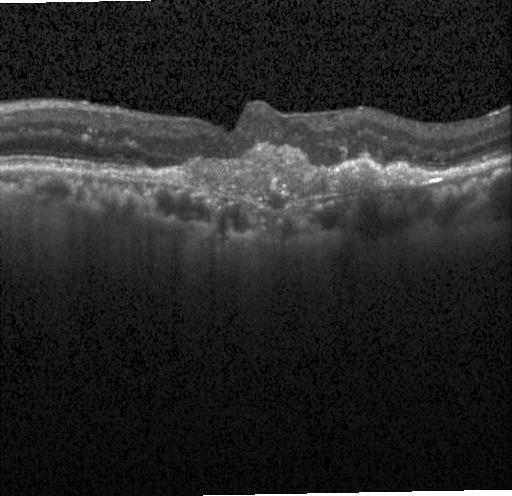
Spectral-domain optical coherence tomography; centered on the fovea; optical coherence tomography B-scan
Diagnosis: choroidal neovascularization.